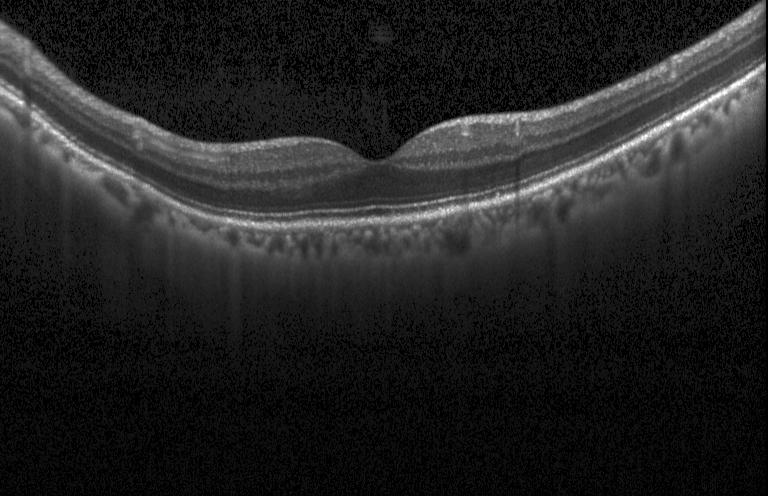

SD-OCT · through the macula · instrument: Heidelberg Spectralis · OCT line scan. This B-scan demonstrates no CNV, DME, or drusen.